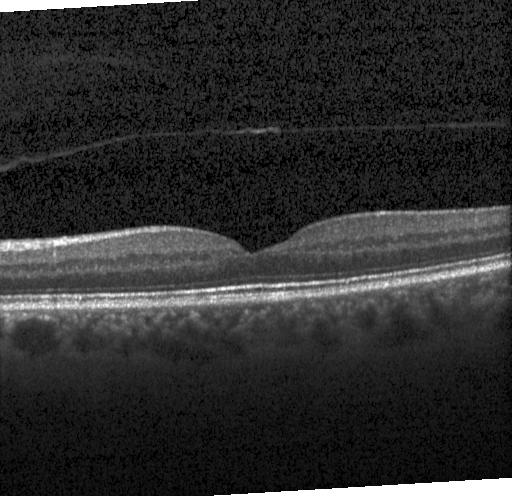 Macular scan. Heidelberg Spectralis. Optical coherence tomography B-scan. SD-OCT
Finding: neither choroidal neovascularization, diabetic macular edema, nor drusen.